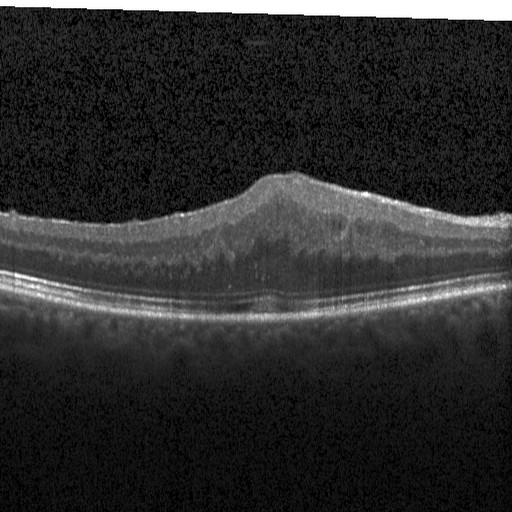 OCT B-scan. Diagnosis: diabetic macular edema (DME).